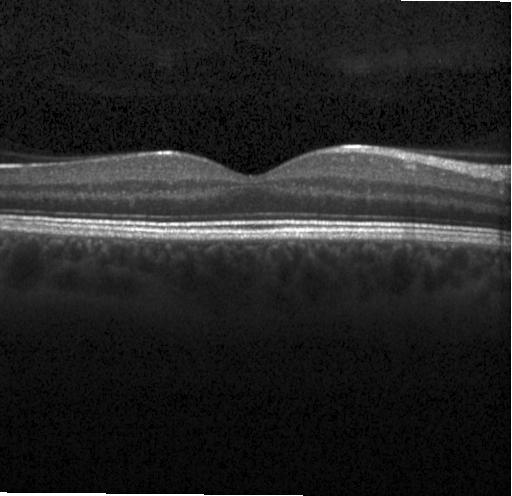
Optical coherence tomography B-scan; through the macula. Impression: no evidence of choroidal neovascularization, diabetic macular edema, or drusen.